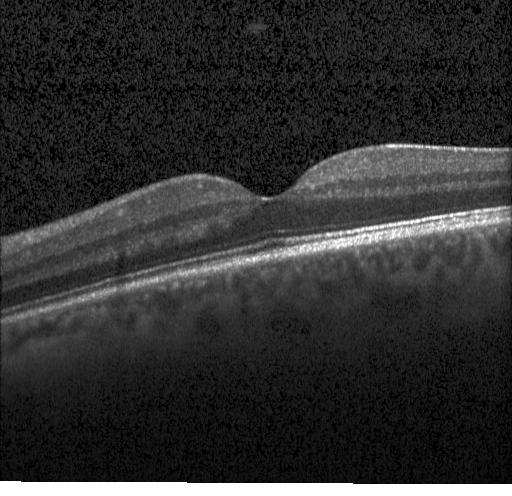

Optical coherence tomography scan, centered on the fovea, spectral-domain optical coherence tomography, acquired on a Heidelberg Spectralis
Macular OCT: no choroidal neovascularization, no diabetic macular edema, and no drusen.